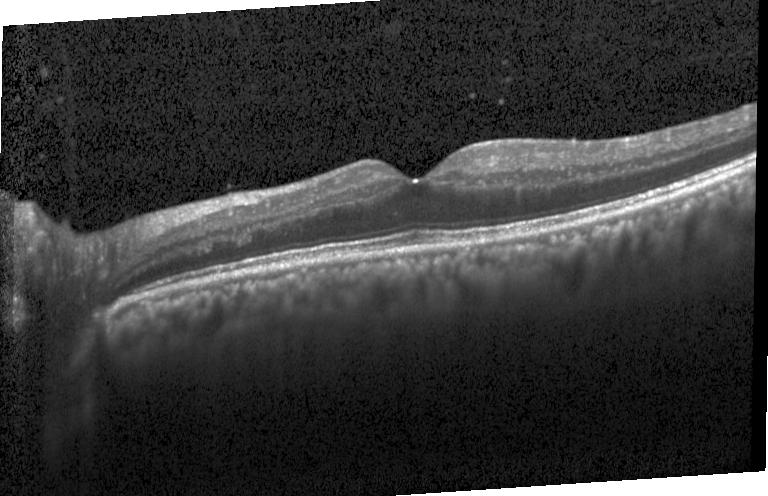
Macular scan. SD-OCT. OCT line scan. Impression: no evidence of CNV, DME, or drusen.